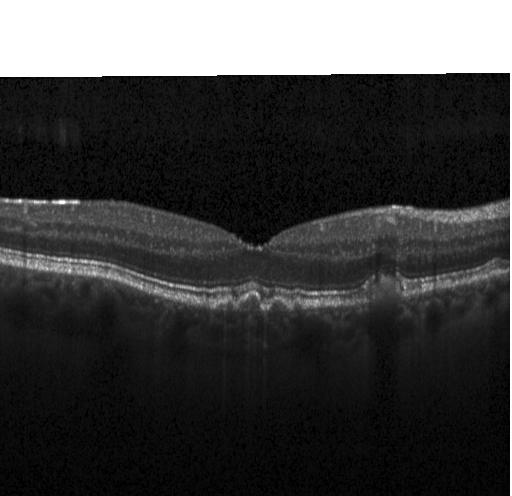

Optical coherence tomography B-scan.
Impression: a choroidal neovascular membrane.